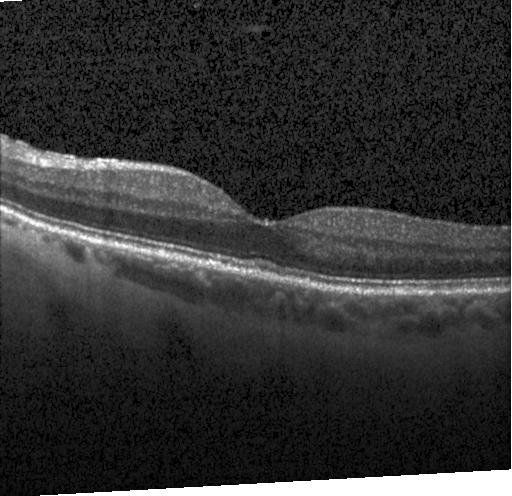

Instrument: Heidelberg Spectralis; horizontal scan through the fovea; spectral-domain OCT; retinal OCT cross-section — Finding: no CNV, DME, or drusen.